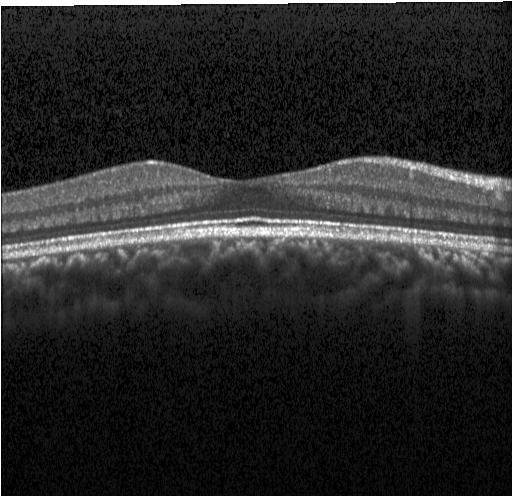

Finding: no evidence of CNV, DME, or drusen.